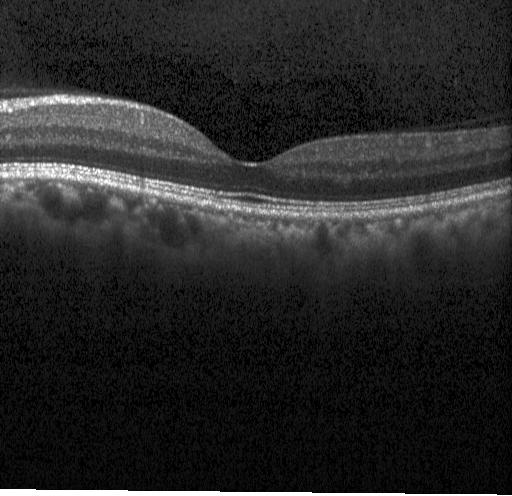
Assessment: neither choroidal neovascularization, diabetic macular edema, nor drusen.